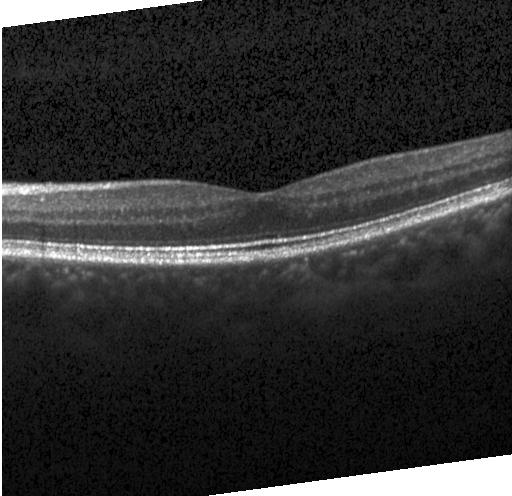

Macular OCT: neither CNV, DME, nor drusen.